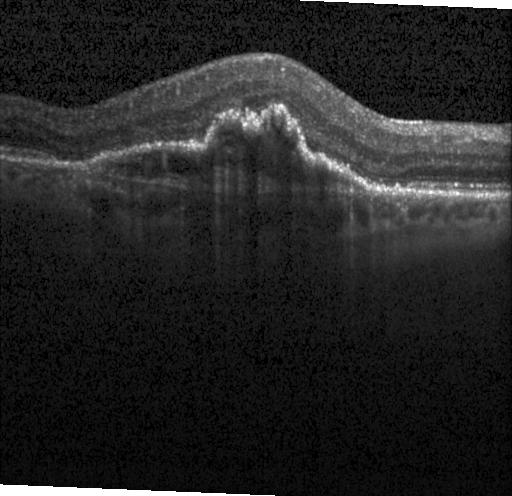 Retinal OCT cross-section.
The scan shows choroidal neovascularization (CNV).